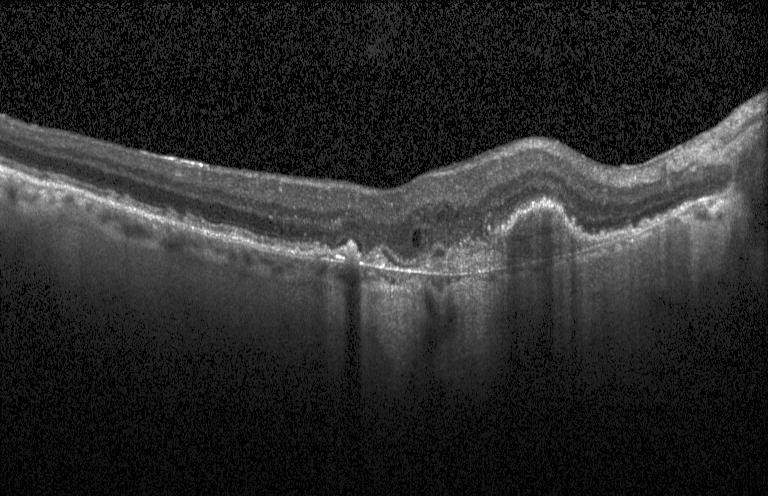 Retinal OCT cross-section. Assessment: choroidal neovascularization.